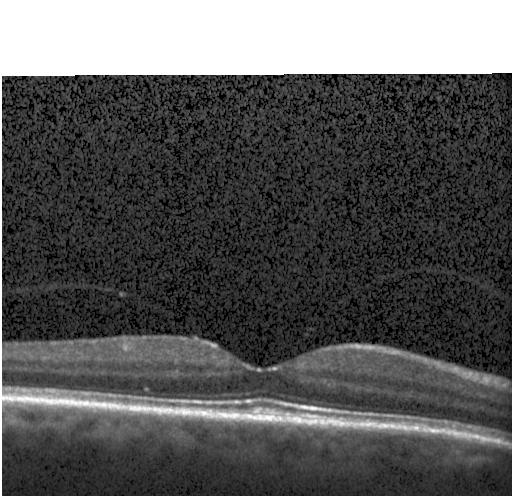
Spectral-domain OCT B-scan: neither choroidal neovascularization, diabetic macular edema, nor drusen.